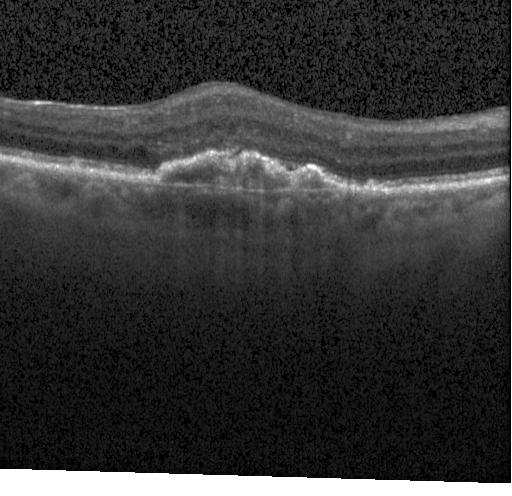 Impression: a choroidal neovascular membrane.